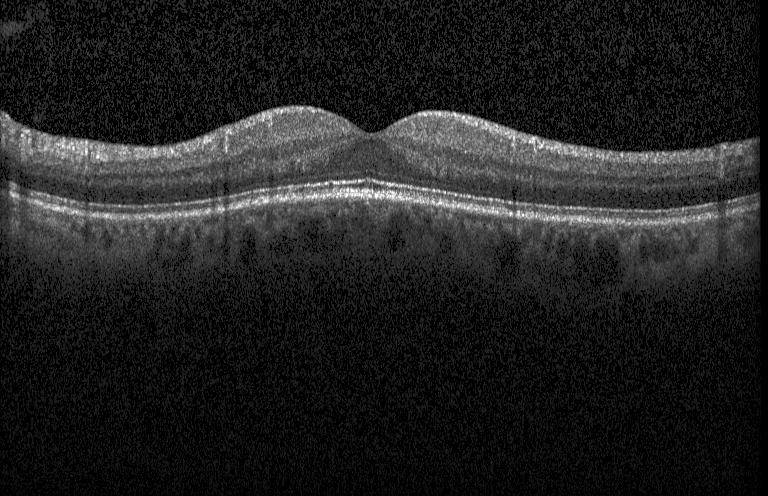 Impression: neither CNV, DME, nor drusen.